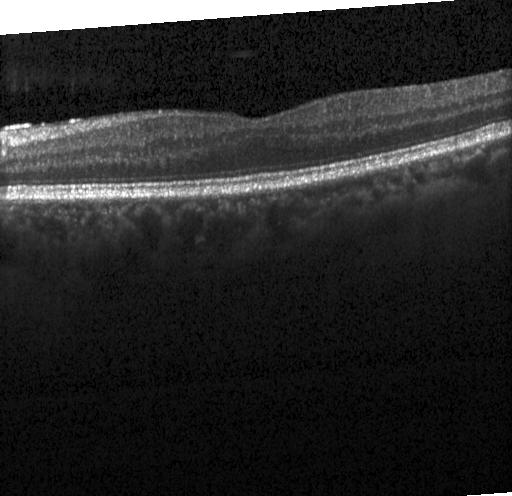 Retinal OCT B-scan
Diagnosis: no choroidal neovascularization, no diabetic macular edema, and no drusen.